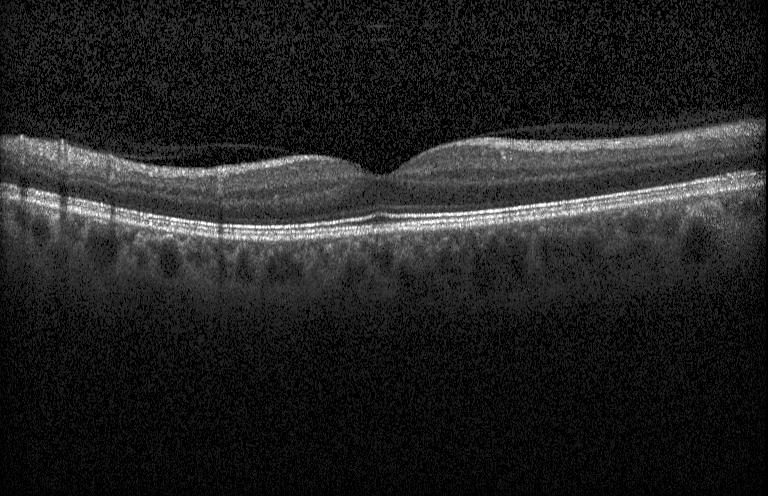

Diagnosis: no evidence of CNV, DME, or drusen.